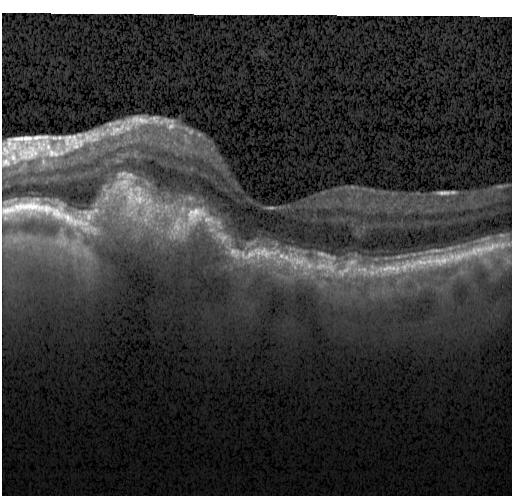 Impression: a choroidal neovascular membrane.